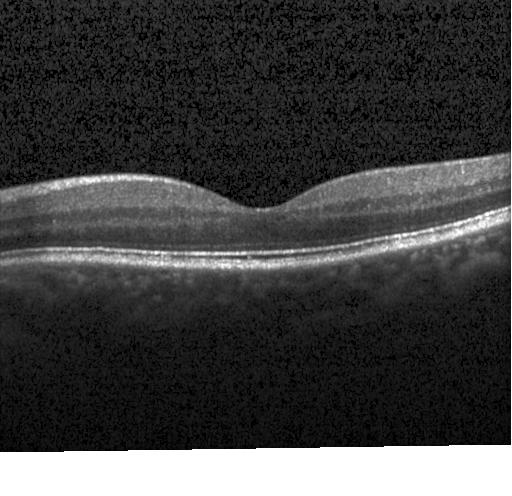 Acquired on a Heidelberg Spectralis. SD-OCT. Retinal OCT cross-section. OCT finding: no choroidal neovascularization, no diabetic macular edema, and no drusen.